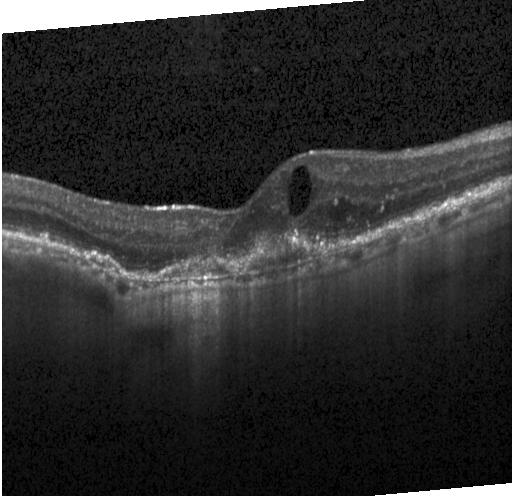

Spectral-domain OCT. Optical coherence tomography B-scan. Finding: CNV.